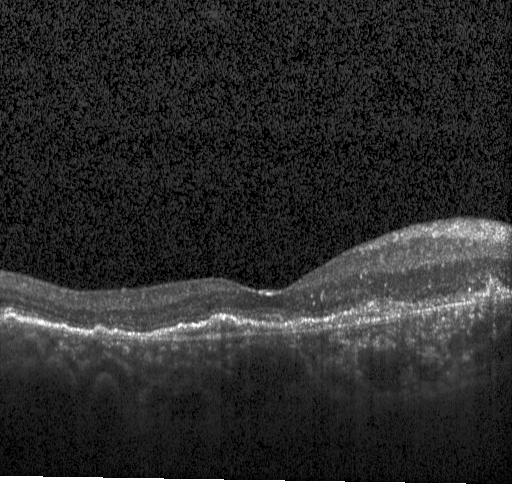 This B-scan demonstrates CNV.